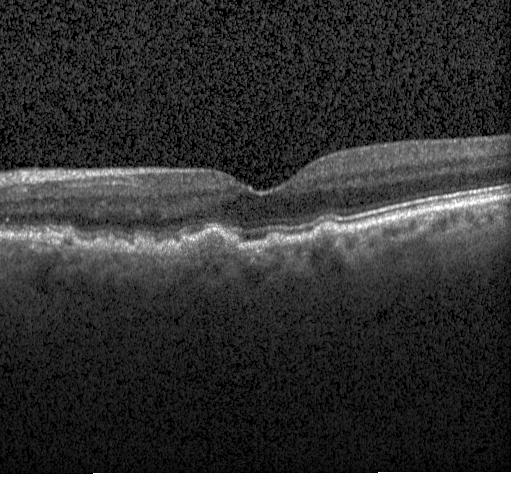

Optical coherence tomography scan · Heidelberg Spectralis OCT system · through the macula.
Dx: multiple drusen.